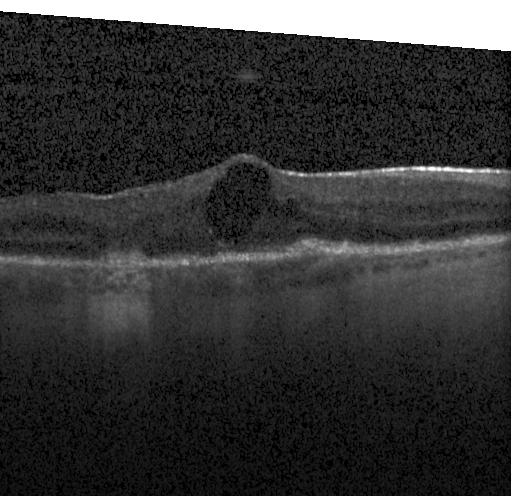 Spectral-domain optical coherence tomography; OCT line scan; macular scan.
Impression: choroidal neovascularization.